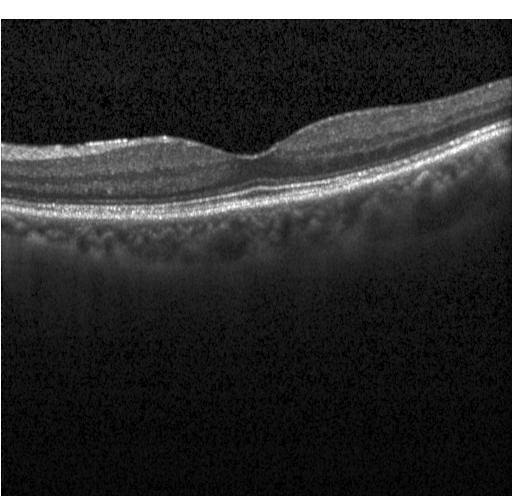

Assessment: neither choroidal neovascularization, diabetic macular edema, nor drusen.